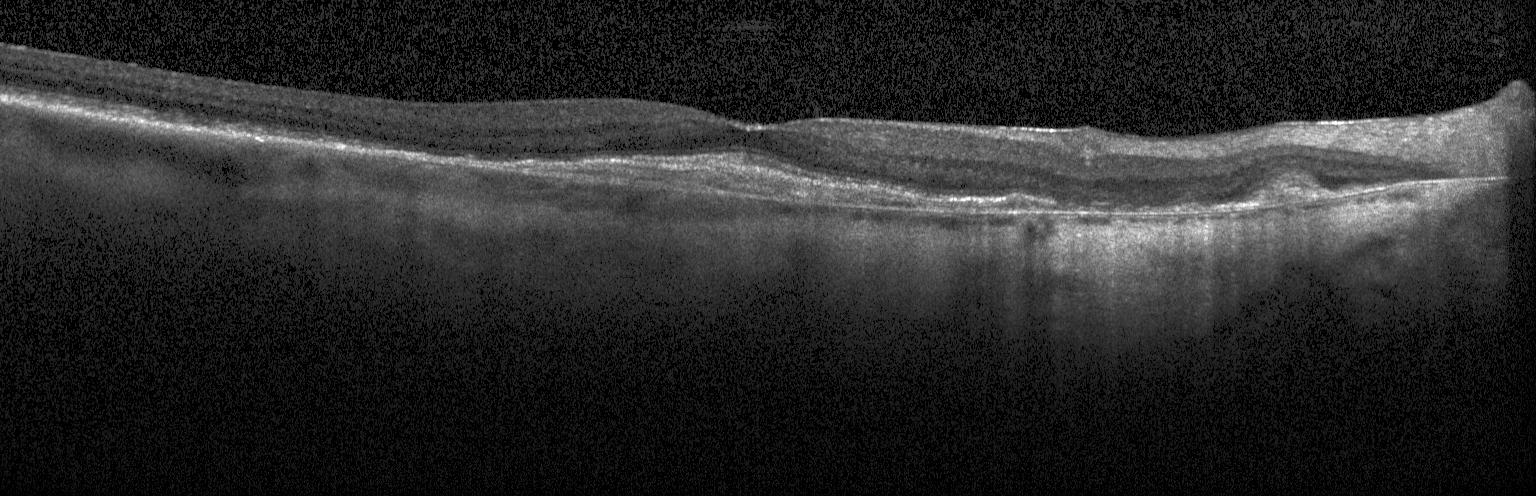

Spectral-domain optical coherence tomography · centered on the fovea · retinal OCT B-scan · Heidelberg Spectralis OCT system
This B-scan demonstrates a choroidal neovascular membrane.